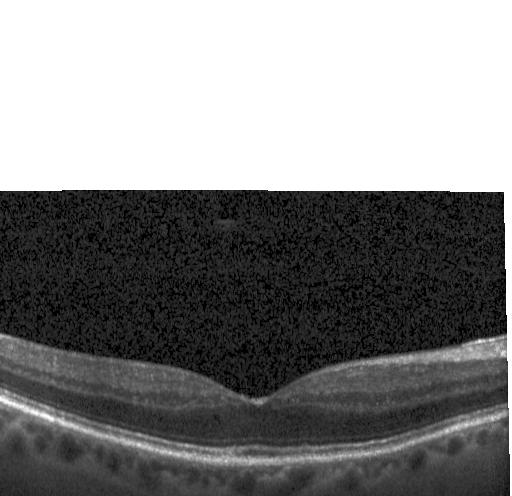
Spectral-domain OCT B-scan: no evidence of choroidal neovascularization, diabetic macular edema, or drusen.